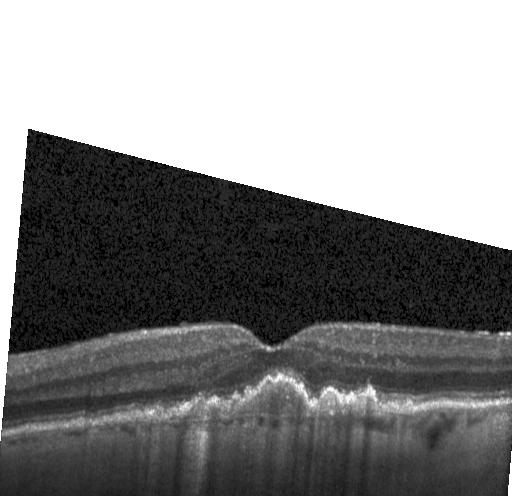 Macular OCT demonstrating choroidal neovascularization (CNV).